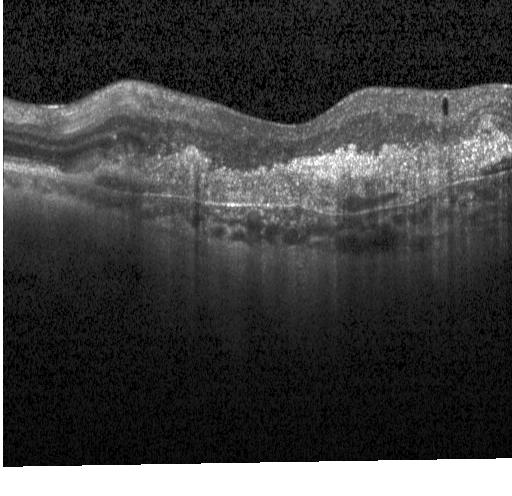
OCT B-scan. OCT finding: a choroidal neovascular membrane.